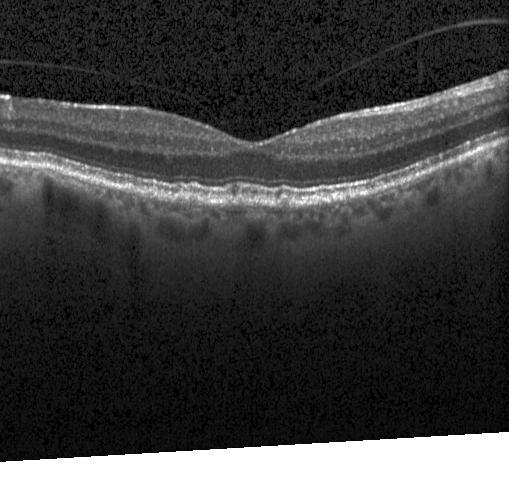

Horizontal scan through the fovea, OCT line scan, spectral-domain OCT, acquired on a Heidelberg Spectralis
The scan shows multiple drusen.